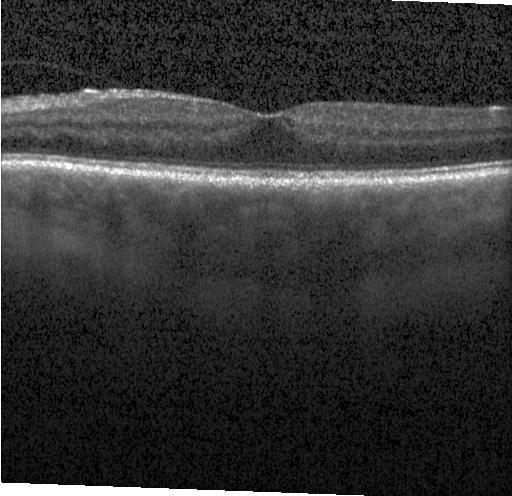 Finding: neither choroidal neovascularization, diabetic macular edema, nor drusen.